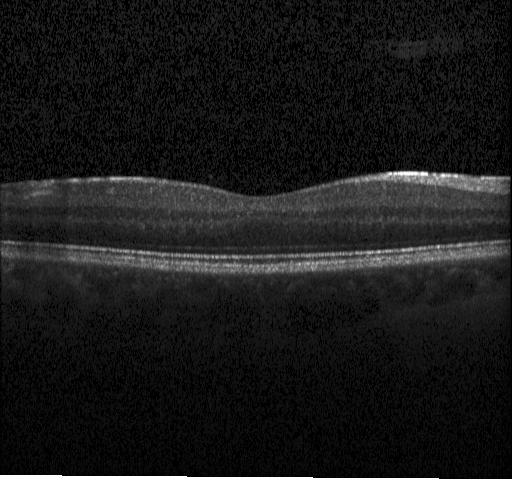

Dx: no choroidal neovascularization, diabetic macular edema, or drusen.